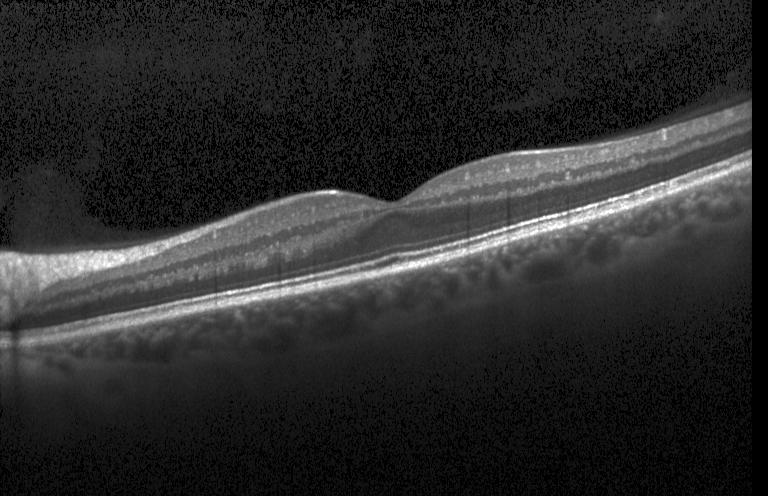
OCT B-scan · acquired on a Heidelberg Spectralis · SD-OCT. Impression: no CNV, no DME, and no drusen.